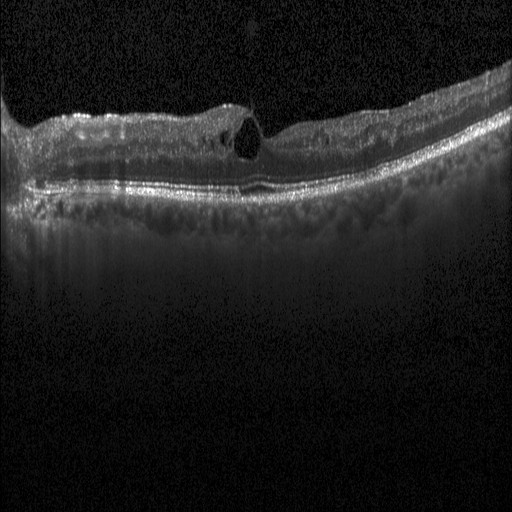 Dx: diabetic macular edema (DME).